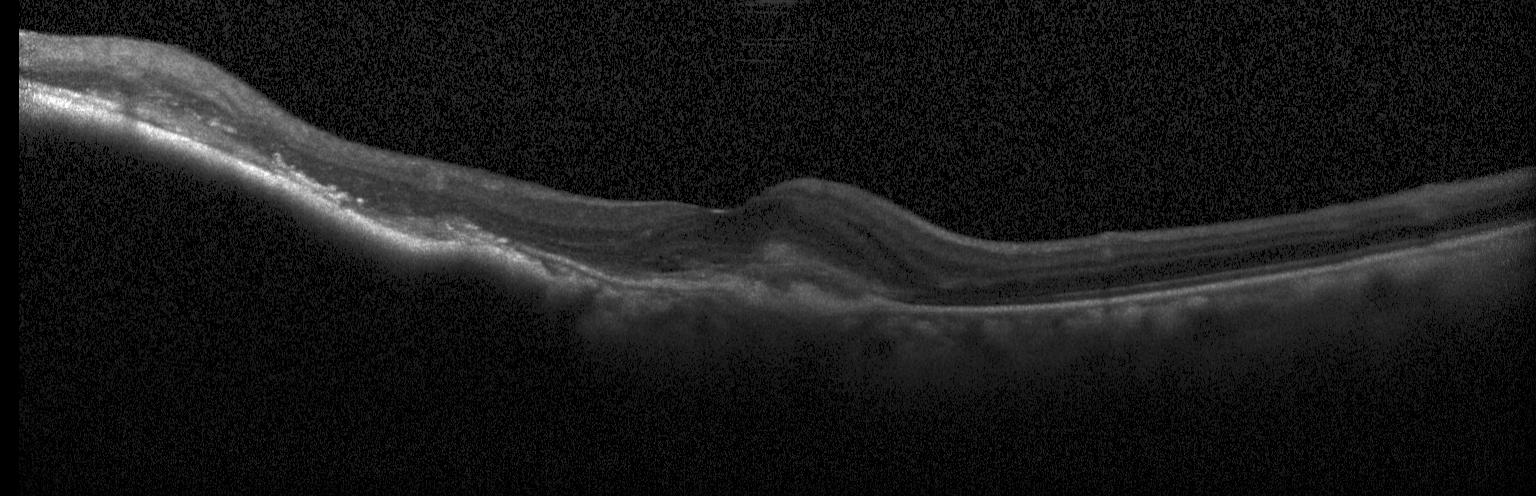
Diagnosis: a choroidal neovascular membrane.